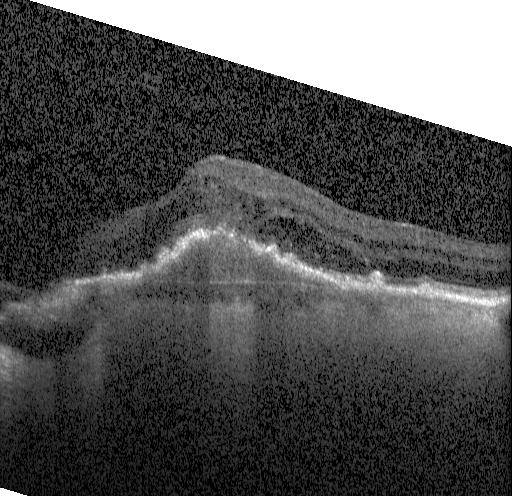

Acquired on a Heidelberg Spectralis. Retinal OCT cross-section. Through the macula. Spectral-domain optical coherence tomography — OCT finding: choroidal neovascularization.